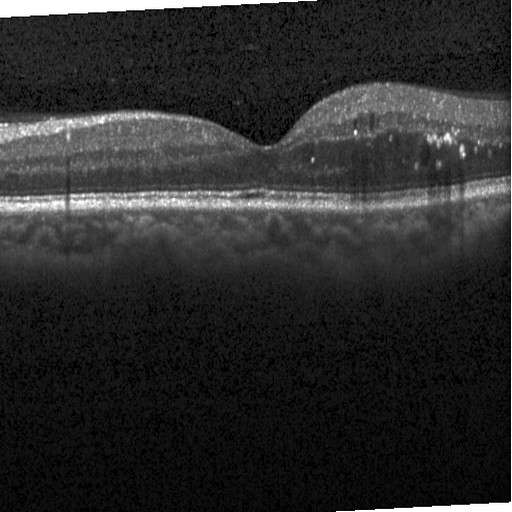
Heidelberg Spectralis OCT system · spectral-domain OCT · optical coherence tomography B-scan · centered on the fovea — Finding: diabetic macular edema.